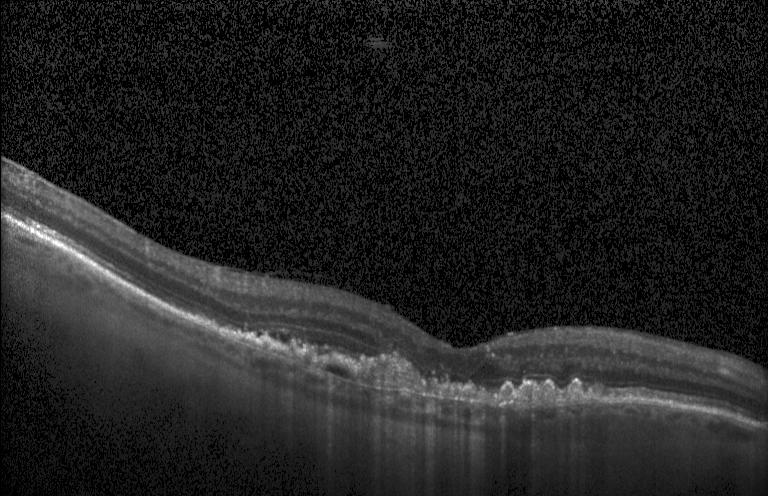

Heidelberg Spectralis. Spectral-domain optical coherence tomography. Retinal OCT cross-section. Centered on the fovea. Finding: a choroidal neovascular membrane.